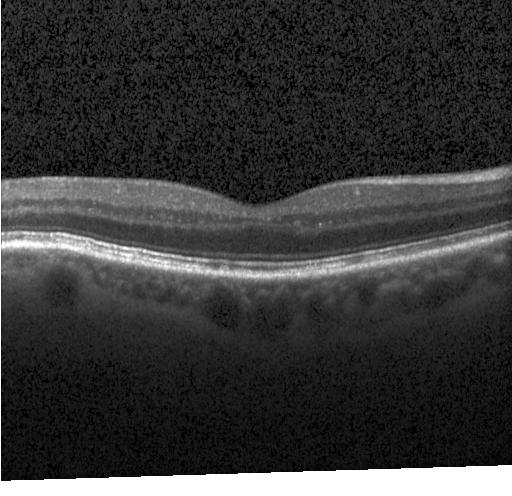
Diagnosis: no choroidal neovascularization, no diabetic macular edema, and no drusen.